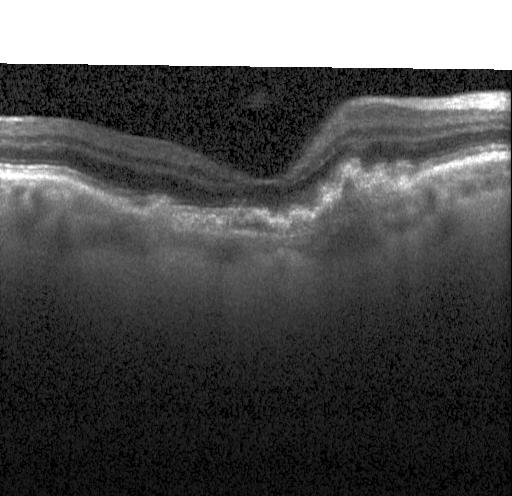 OCT B-scan. Diagnosis: a choroidal neovascular membrane.